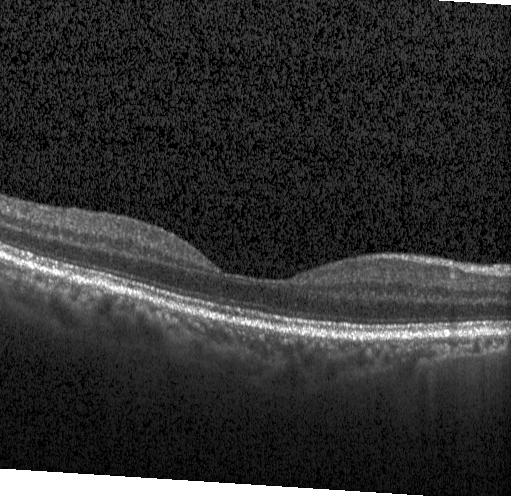
OCT B-scan; fovea-centered; Heidelberg Spectralis.
Finding: no CNV, DME, or drusen.